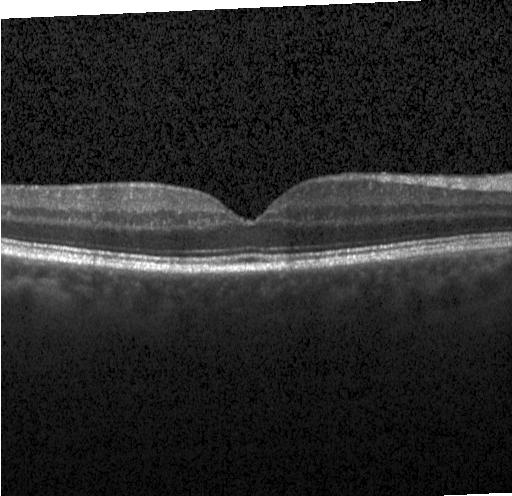
Impression: no evidence of CNV, DME, or drusen.